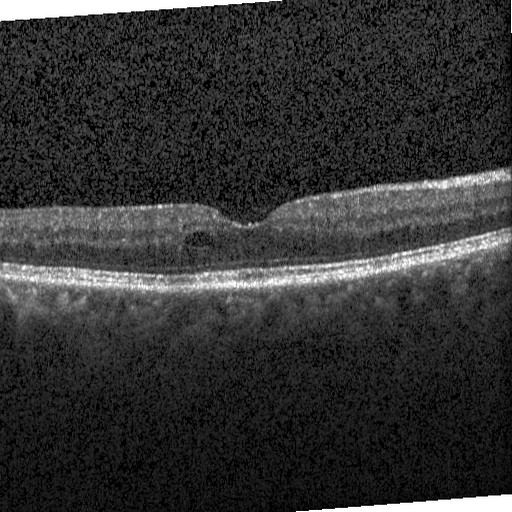 Heidelberg Spectralis. SD-OCT. Optical coherence tomography B-scan — The scan shows diabetic macular edema (DME).